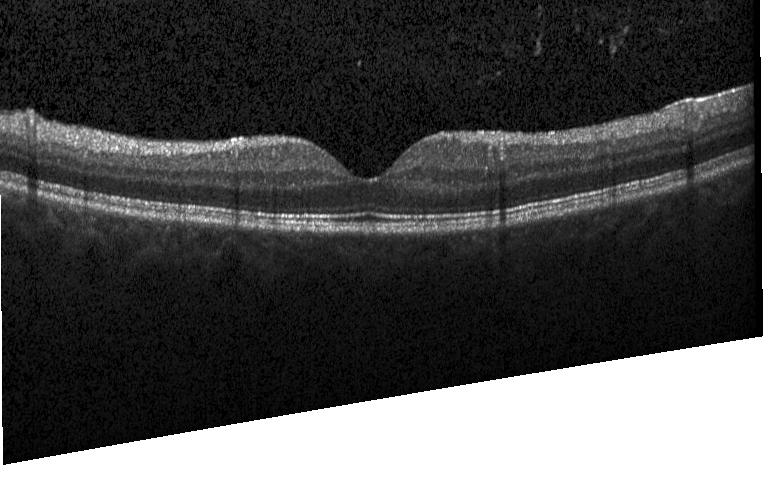 Retinal OCT cross-section showing no CNV, DME, or drusen.